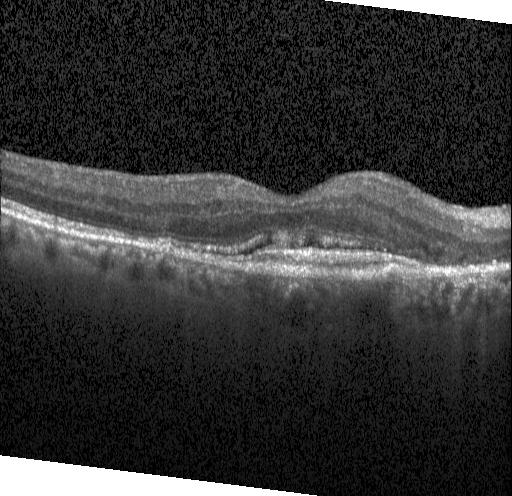

Centered on the fovea, SD-OCT, instrument: Heidelberg Spectralis, retinal OCT cross-section.
Finding: choroidal neovascularization (CNV).